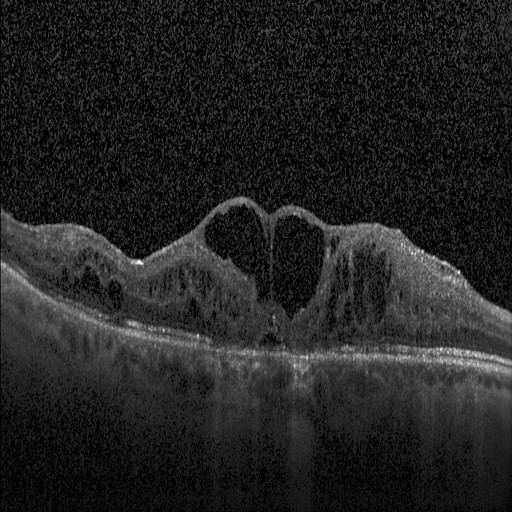 Finding: DME.